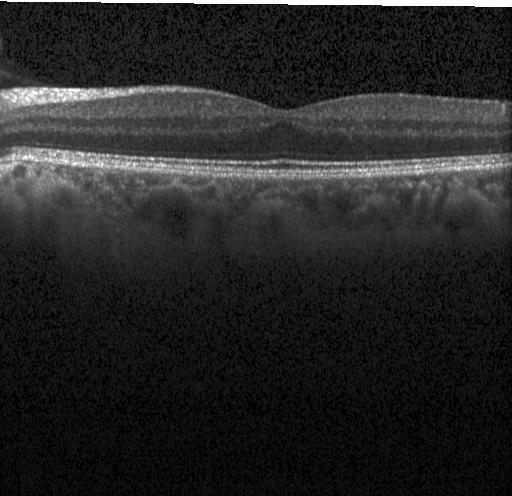

OCT line scan · acquired on a Heidelberg Spectralis. Diagnosis: no evidence of choroidal neovascularization, diabetic macular edema, or drusen.